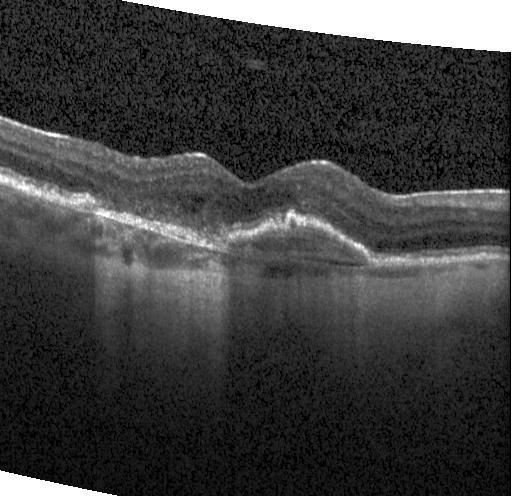 Spectral-domain OCT B-scan: a choroidal neovascular membrane.